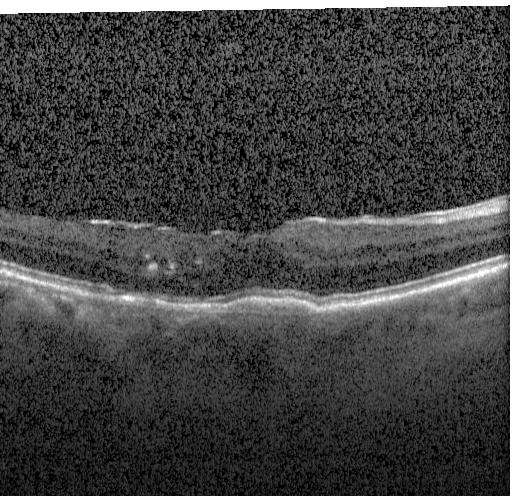 Retinal OCT B-scan · spectral-domain optical coherence tomography · through the macula. Impression: a choroidal neovascular membrane.